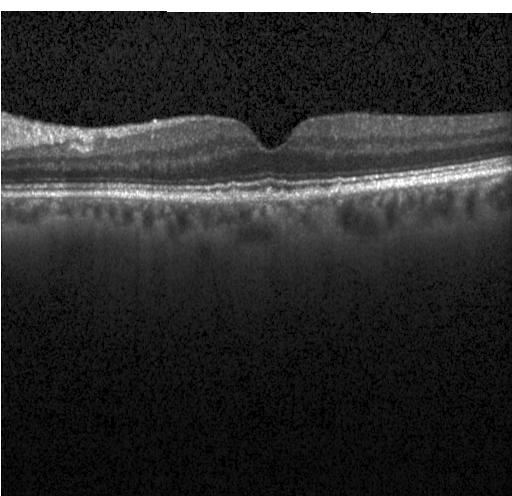

Retinal OCT B-scan.
Assessment: sub-RPE drusenoid deposits.